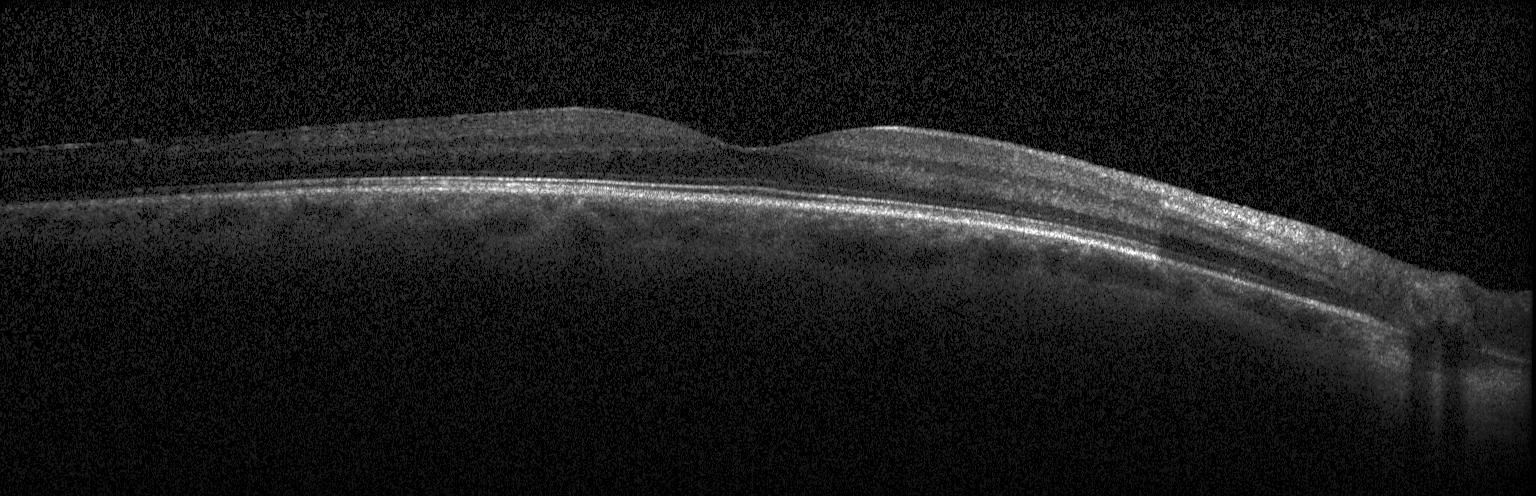
Centered on the fovea; Heidelberg Spectralis; spectral-domain OCT; optical coherence tomography B-scan.
No choroidal neovascularization, diabetic macular edema, or drusen.